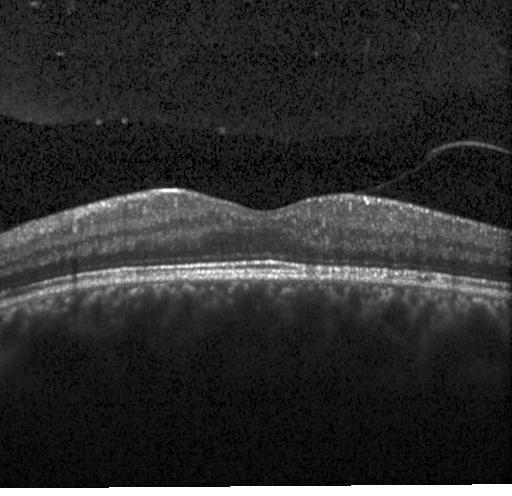
Finding: no choroidal neovascularization, diabetic macular edema, or drusen.